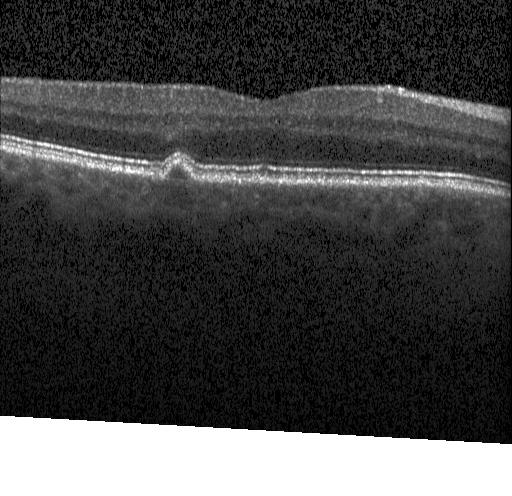 Finding: multiple drusen.